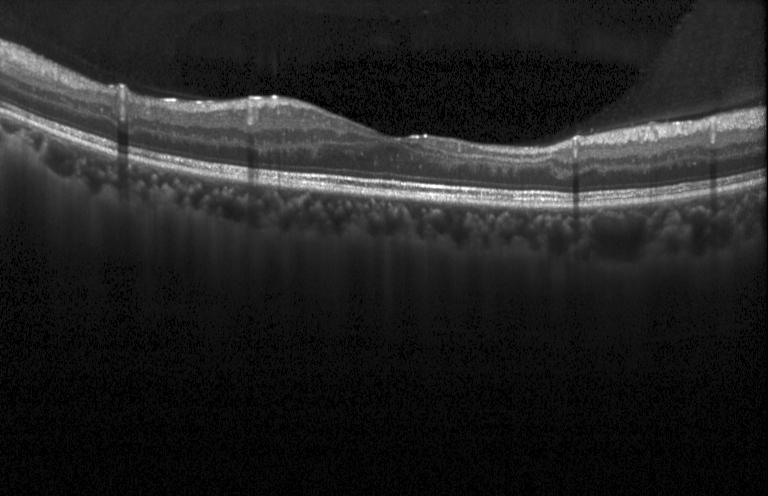 Spectral-domain OCT; retinal OCT B-scan. Finding: no evidence of CNV, DME, or drusen.